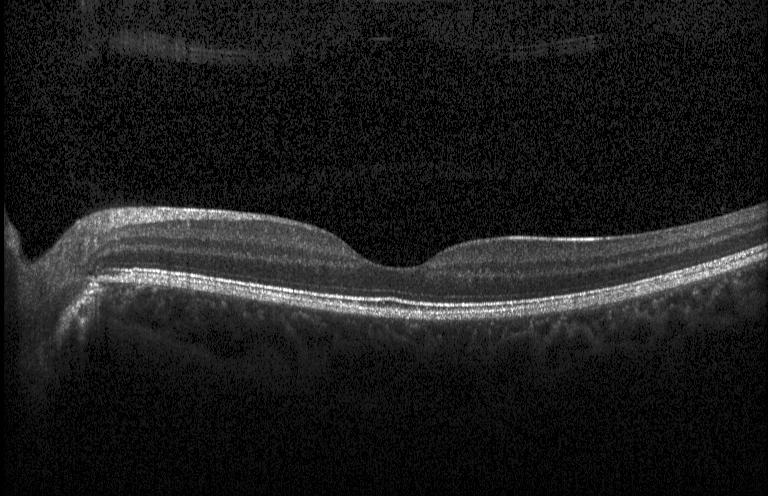 Optical coherence tomography scan. Assessment: no choroidal neovascularization, diabetic macular edema, or drusen.